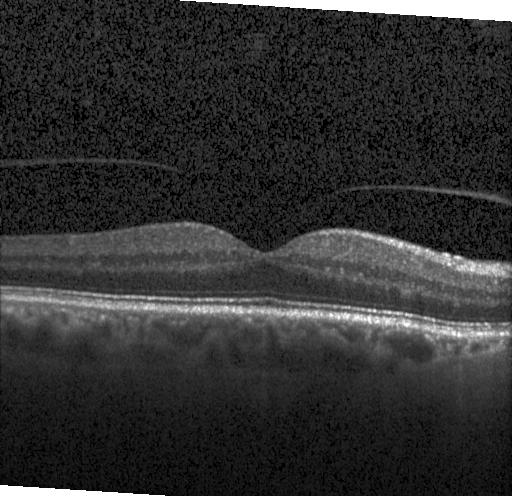

SD-OCT; fovea-centered; retinal OCT cross-section; acquired on a Heidelberg Spectralis — Finding: no evidence of choroidal neovascularization, diabetic macular edema, or drusen.